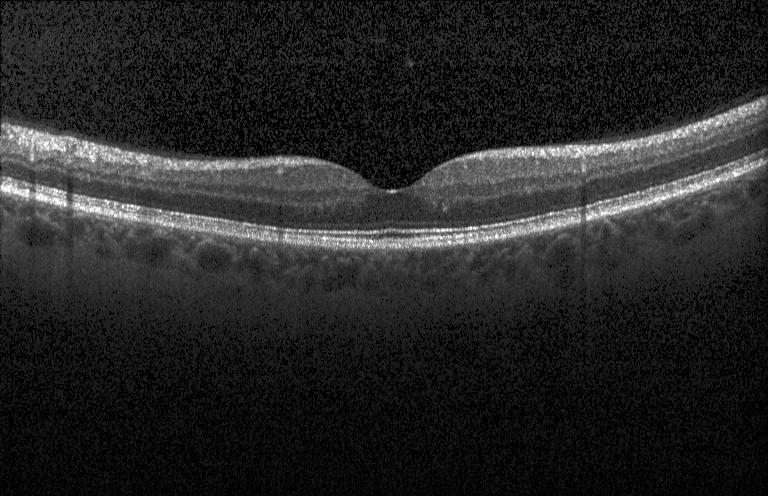

No choroidal neovascularization, diabetic macular edema, or drusen.